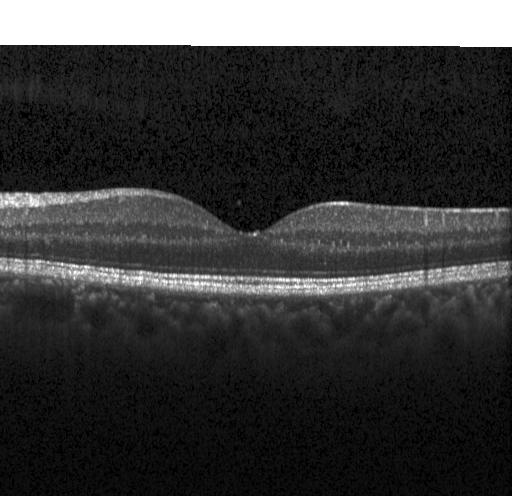

Retinal OCT B-scan — Dx: no CNV, no DME, and no drusen.